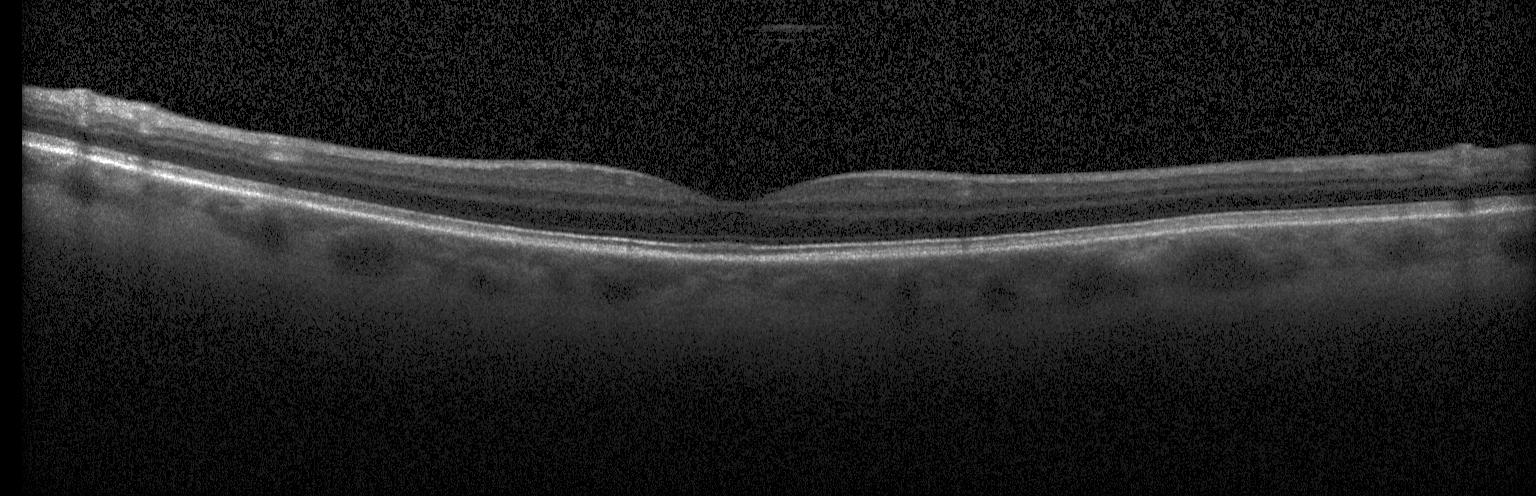
Heidelberg Spectralis OCT system, retinal OCT B-scan, through the macula, spectral-domain optical coherence tomography
Impression: no choroidal neovascularization, no diabetic macular edema, and no drusen.